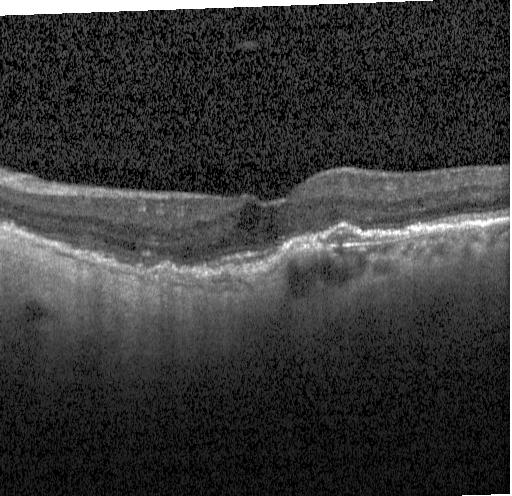 Instrument: Heidelberg Spectralis, OCT B-scan, fovea-centered
The scan shows a choroidal neovascular membrane.